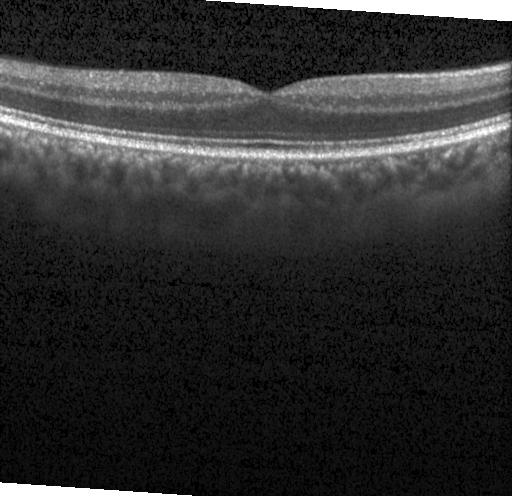
Heidelberg Spectralis; OCT B-scan. Assessment: no evidence of choroidal neovascularization, diabetic macular edema, or drusen.